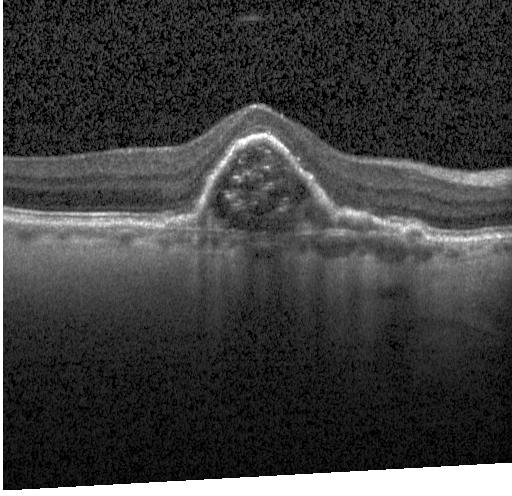
Optical coherence tomography scan · SD-OCT
Diagnosis: a choroidal neovascular membrane.